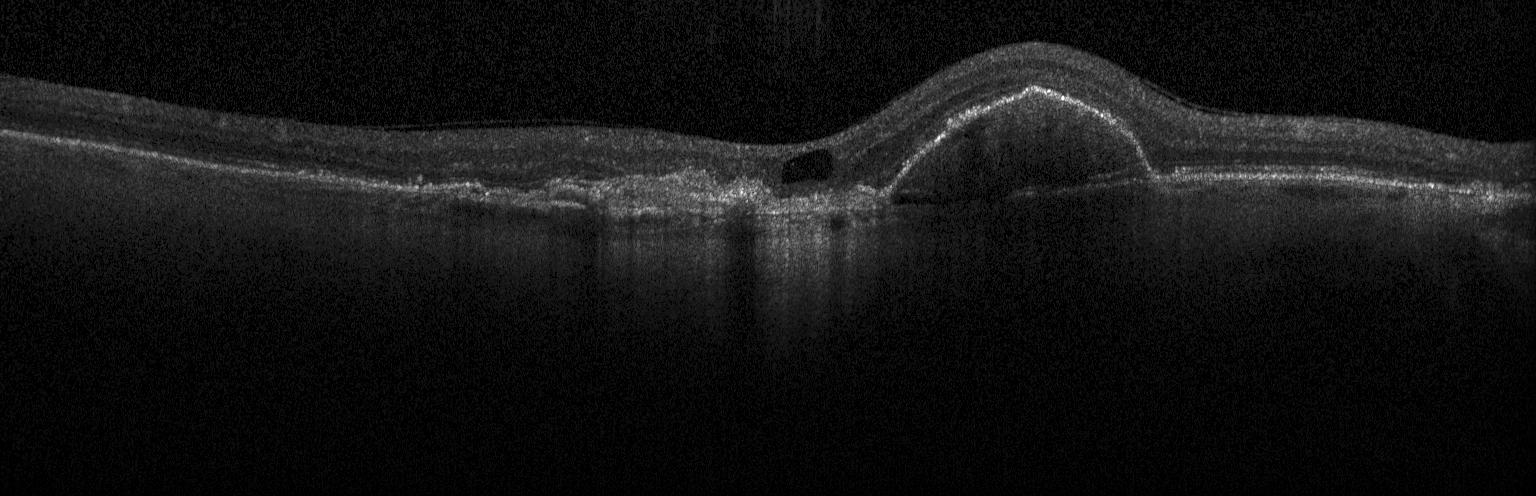

Retinal OCT cross-section, spectral-domain OCT, centered on the fovea — This B-scan demonstrates CNV.